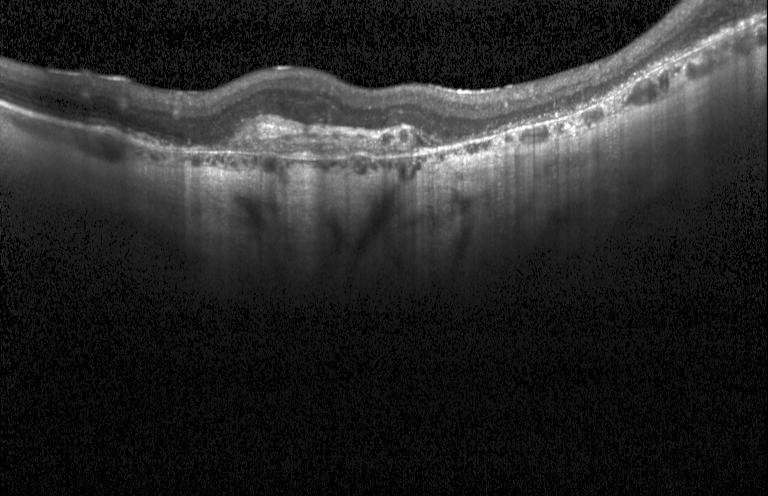
Spectral-domain OCT B-scan: choroidal neovascularization (CNV).